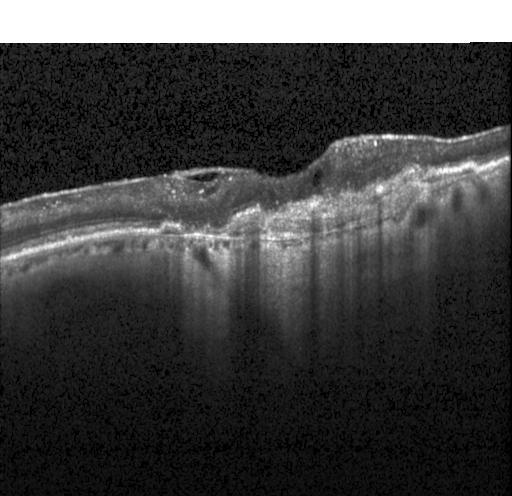

Diagnosis: a choroidal neovascular membrane.